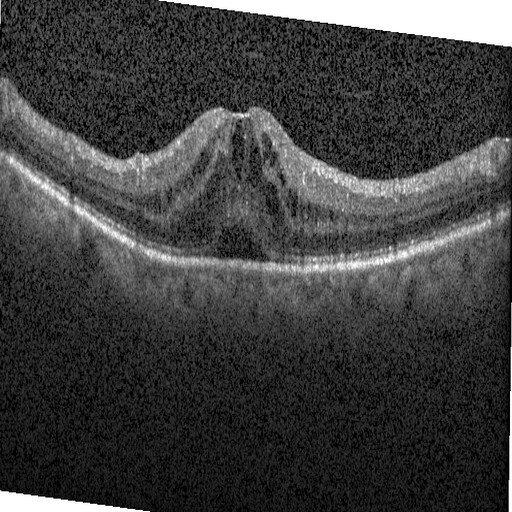 Retinal OCT cross-section.
Finding: DME.